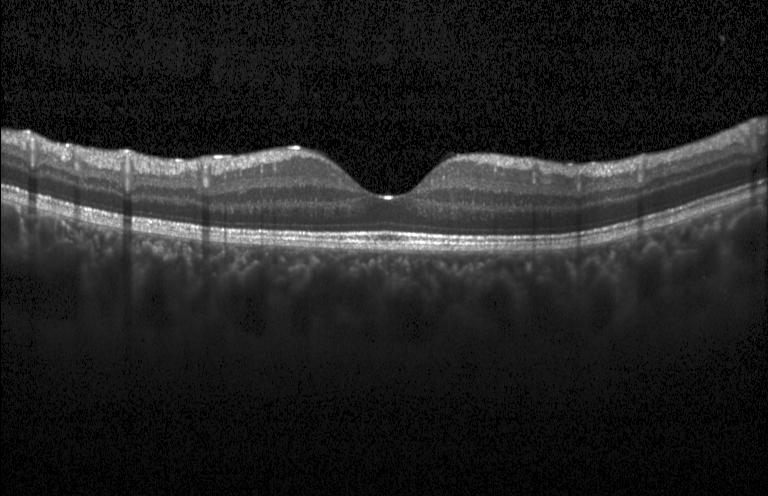 Assessment: neither CNV, DME, nor drusen.